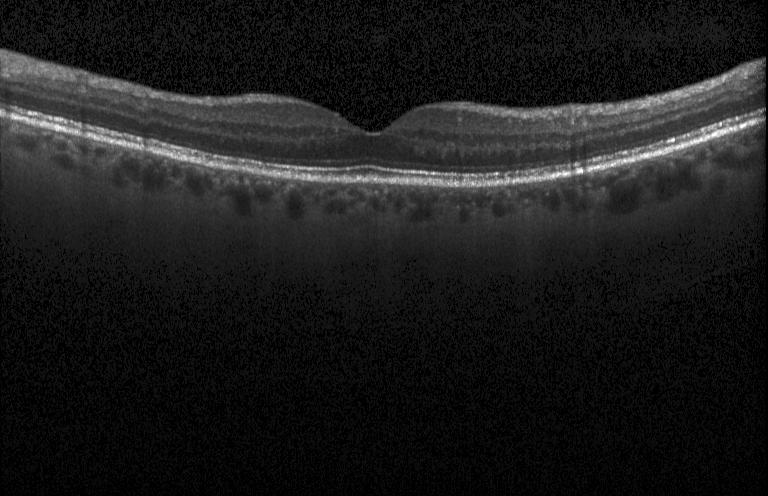
SD-OCT; retinal OCT cross-section; macular scan. Assessment: neither CNV, DME, nor drusen.